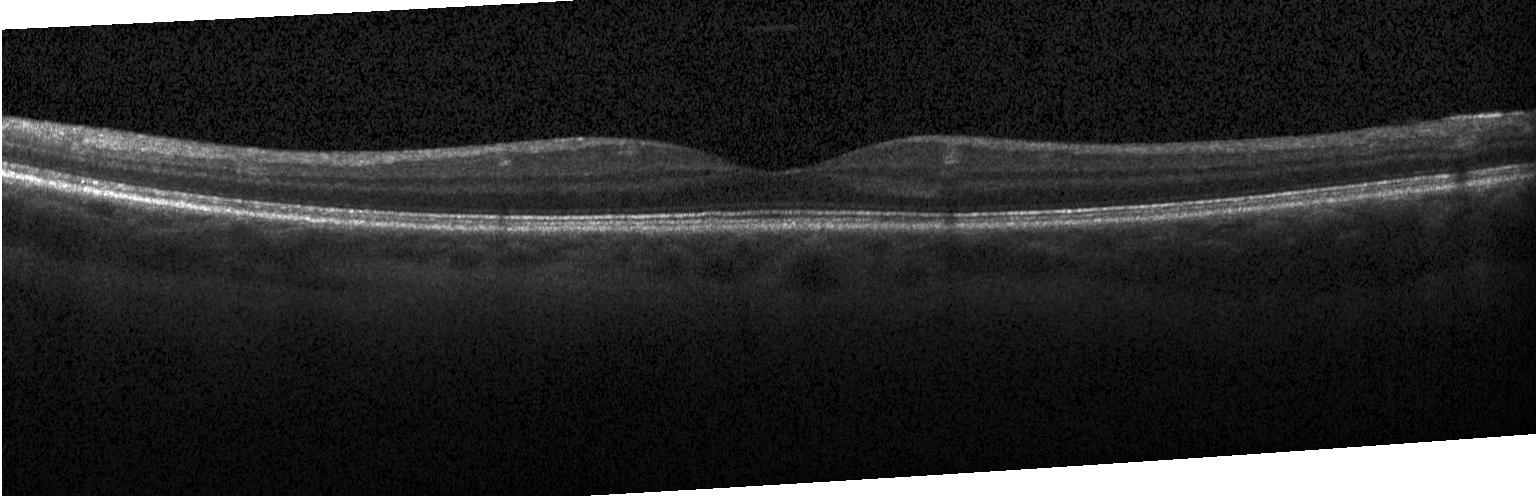

Optical coherence tomography B-scan. Fovea-centered. Instrument: Heidelberg Spectralis. Spectral-domain optical coherence tomography — This B-scan demonstrates neither choroidal neovascularization, diabetic macular edema, nor drusen.